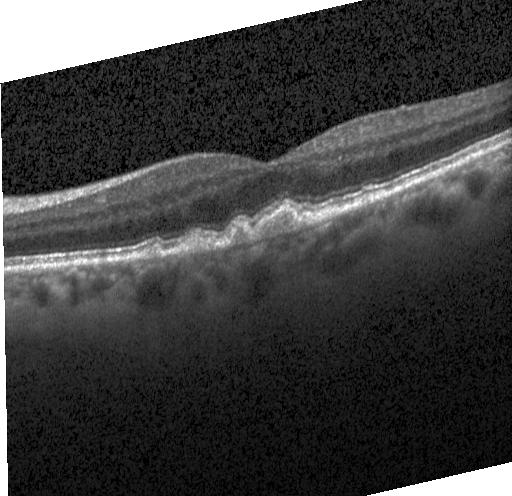 Optical coherence tomography scan, instrument: Heidelberg Spectralis. Drusen.